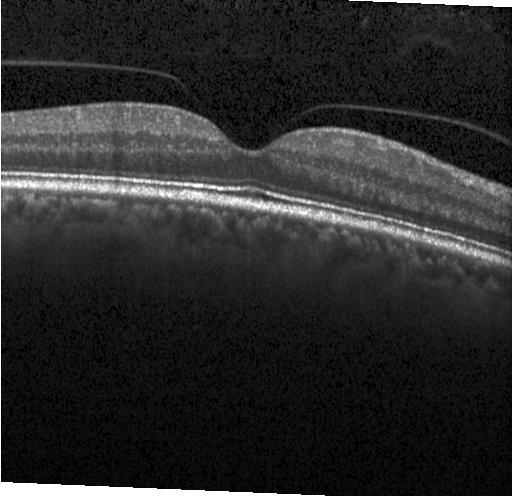

The scan shows no CNV, DME, or drusen.